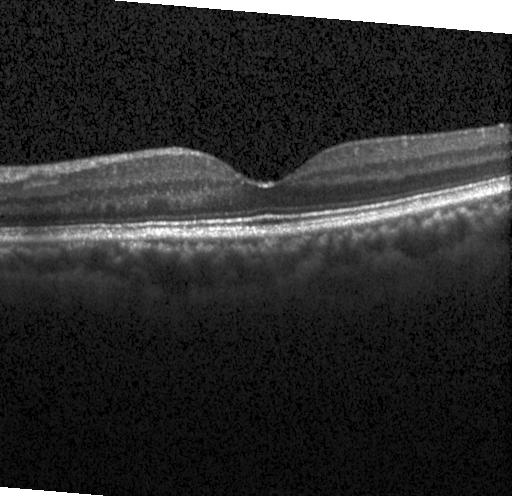
Optical coherence tomography B-scan. Diagnosis: neither CNV, DME, nor drusen.